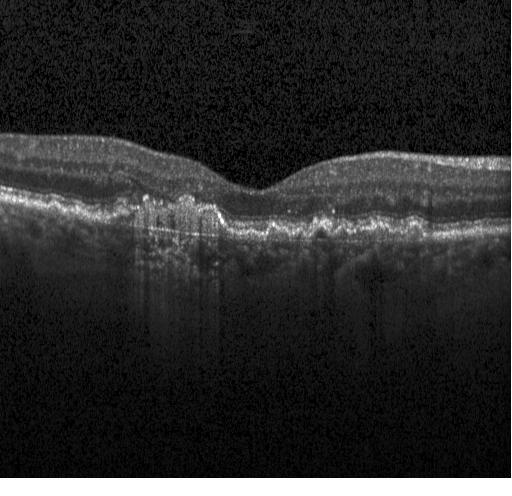
Finding: choroidal neovascularization.